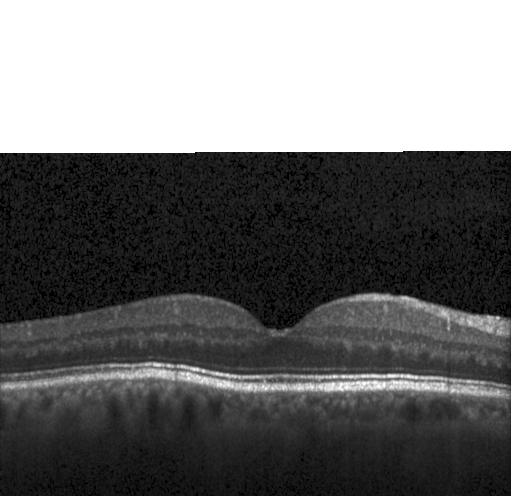 Spectral-domain OCT. Horizontal scan through the fovea. Optical coherence tomography B-scan. No choroidal neovascularization, no diabetic macular edema, and no drusen.